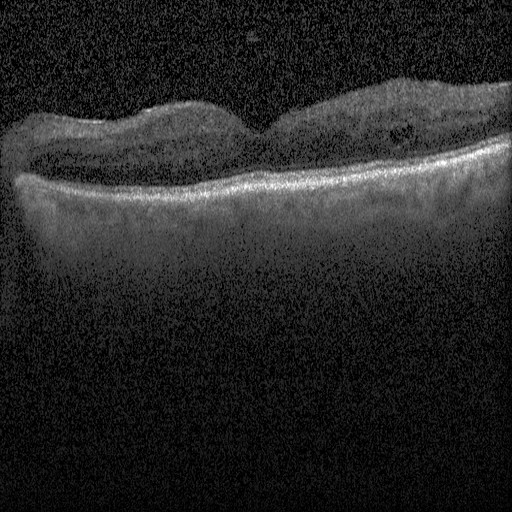 Spectral-domain OCT; instrument: Heidelberg Spectralis; fovea-centered; optical coherence tomography scan. Finding: diabetic macular edema (DME).